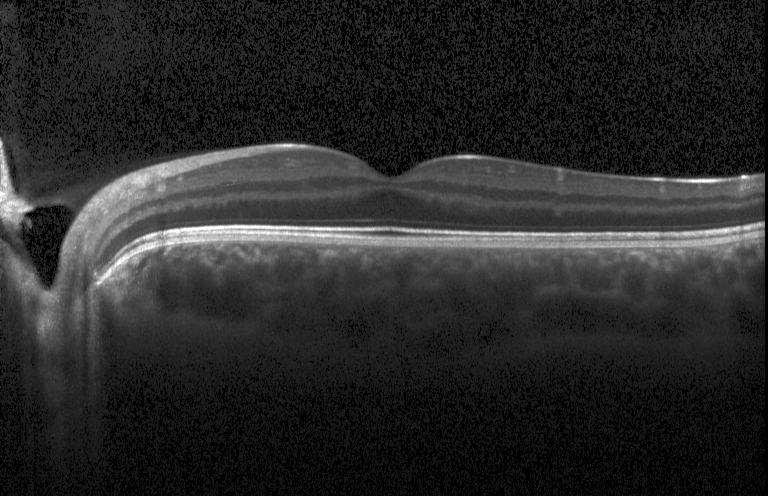 Retinal OCT B-scan · Heidelberg Spectralis OCT system.
Finding: no choroidal neovascularization, diabetic macular edema, or drusen.